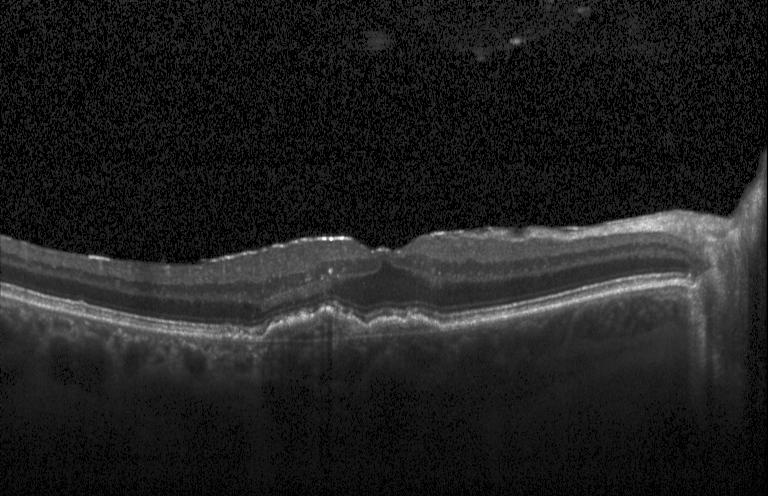 This B-scan demonstrates a choroidal neovascular membrane.